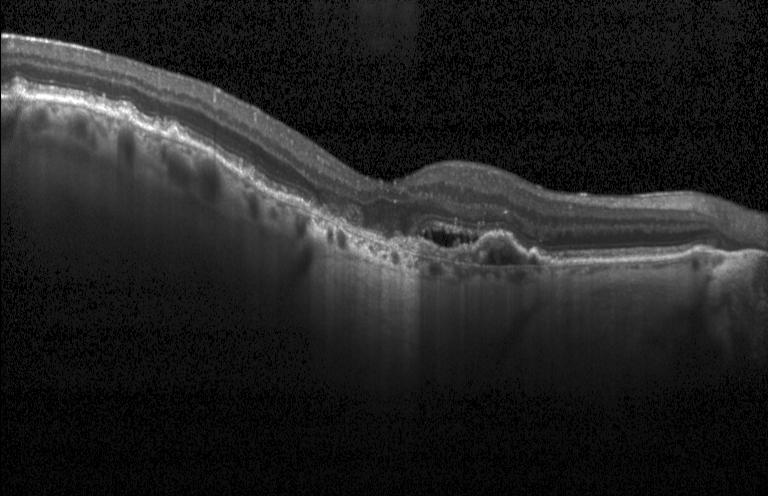 Optical coherence tomography scan — Choroidal neovascularization (CNV).